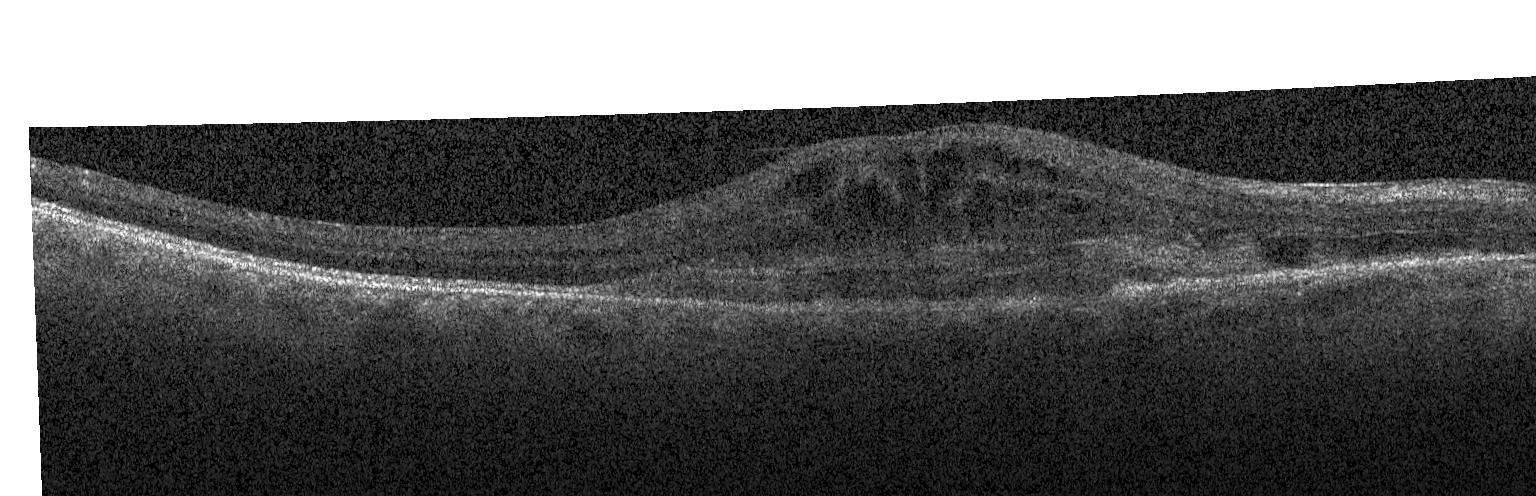

Heidelberg Spectralis OCT system · through the macula · optical coherence tomography scan — Assessment: a choroidal neovascular membrane.